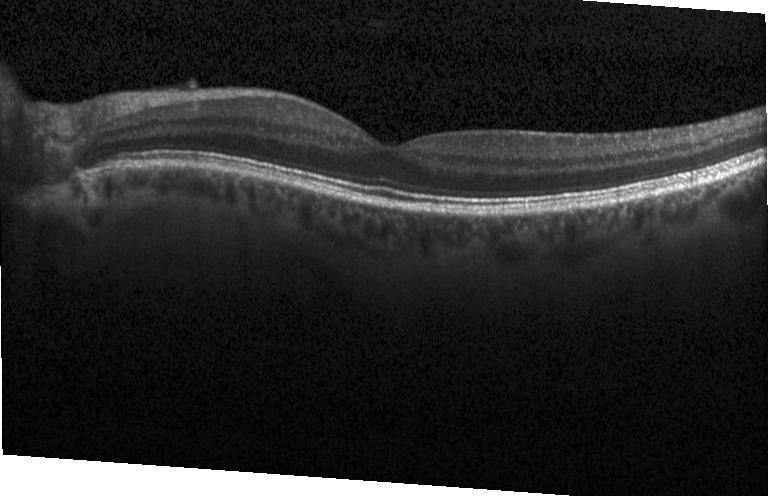

Optical coherence tomography scan, spectral-domain OCT, fovea-centered, Heidelberg Spectralis. Neither CNV, DME, nor drusen.